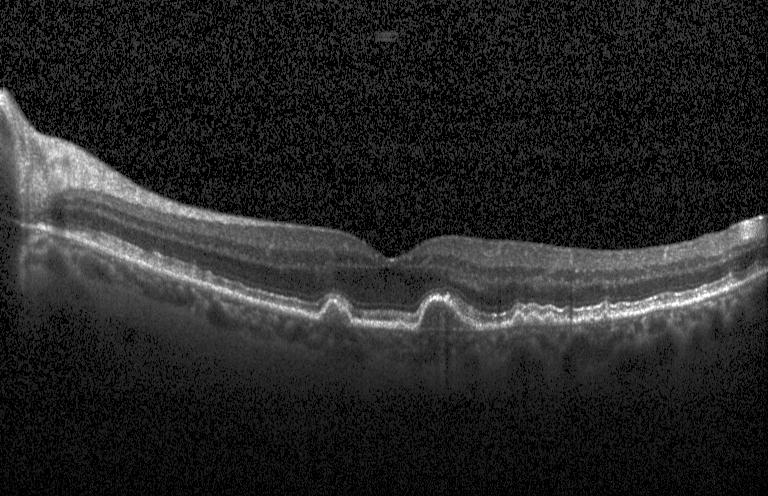 Retinal OCT cross-section showing sub-RPE drusenoid deposits.